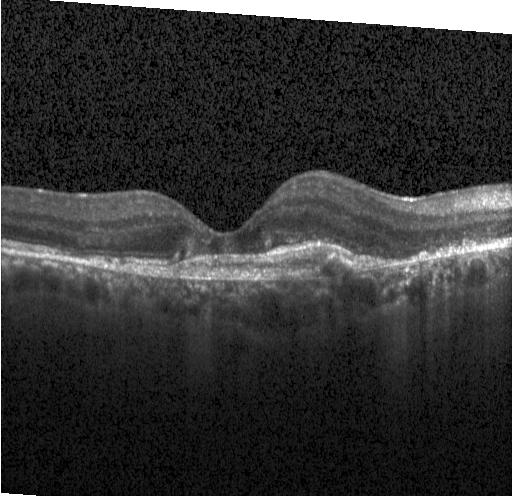
OCT line scan, fovea-centered, Heidelberg Spectralis OCT system.
The scan shows CNV.